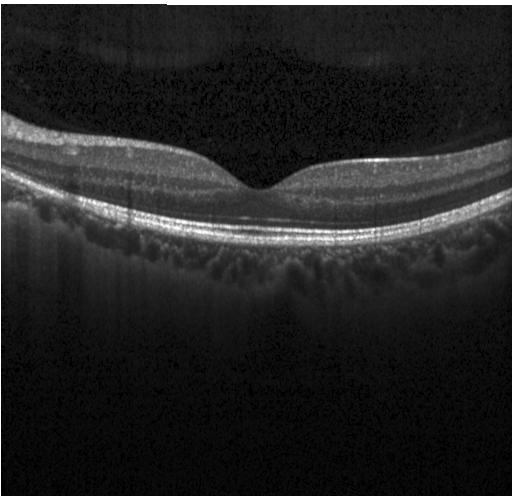
Diagnosis: no choroidal neovascularization, no diabetic macular edema, and no drusen.